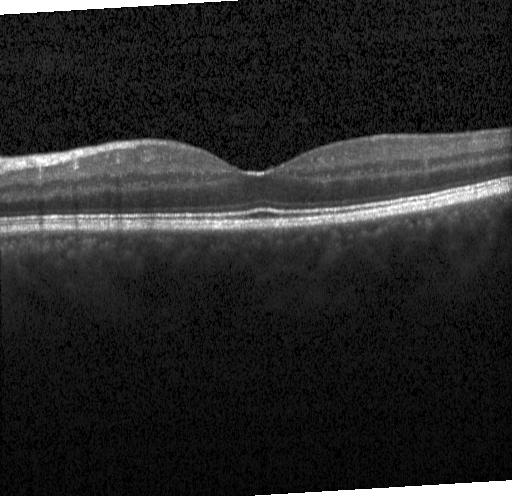 Diagnosis: no choroidal neovascularization, diabetic macular edema, or drusen.